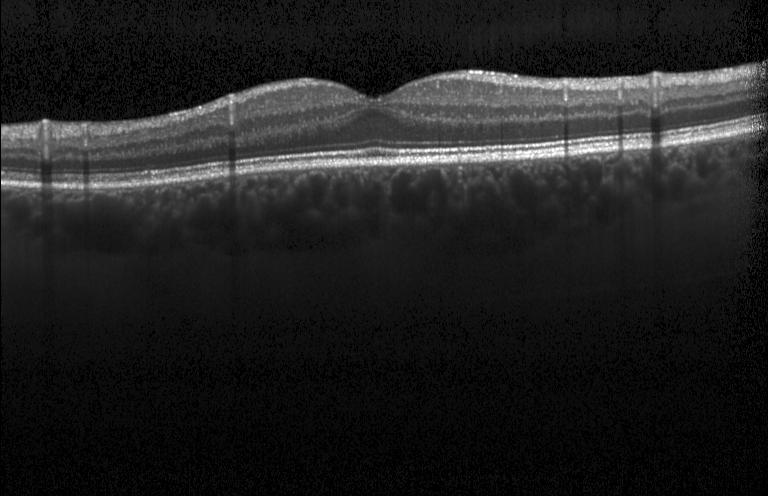
This B-scan demonstrates no choroidal neovascularization, no diabetic macular edema, and no drusen.